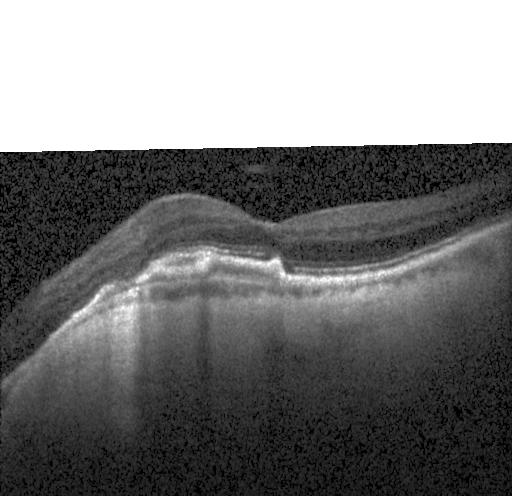

Horizontal scan through the fovea · optical coherence tomography scan — Choroidal neovascularization.